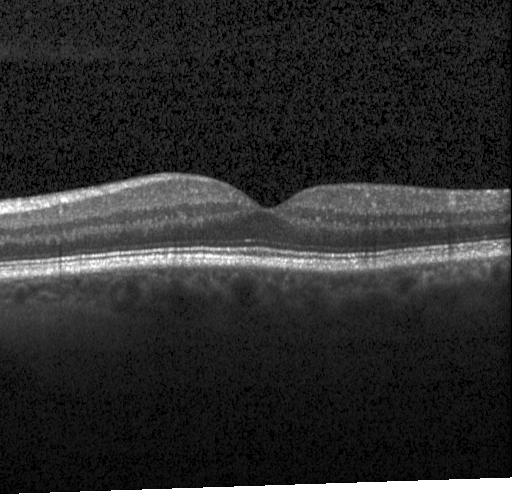
OCT line scan; horizontal scan through the fovea. Diagnosis: no evidence of CNV, DME, or drusen.